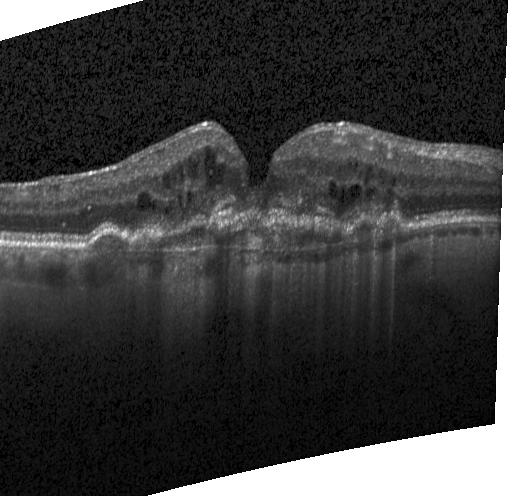

OCT line scan; spectral-domain OCT; acquired on a Heidelberg Spectralis; fovea-centered — Finding: choroidal neovascularization (CNV).